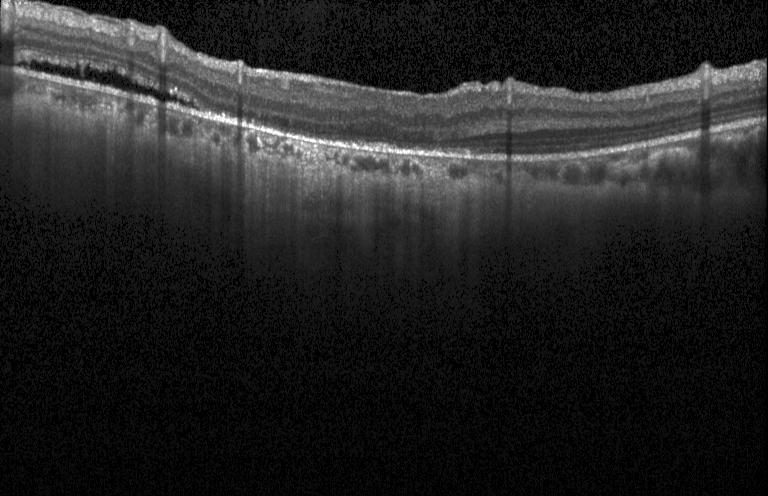
OCT B-scan; Heidelberg Spectralis OCT system; macular scan; spectral-domain optical coherence tomography. The scan shows a choroidal neovascular membrane.